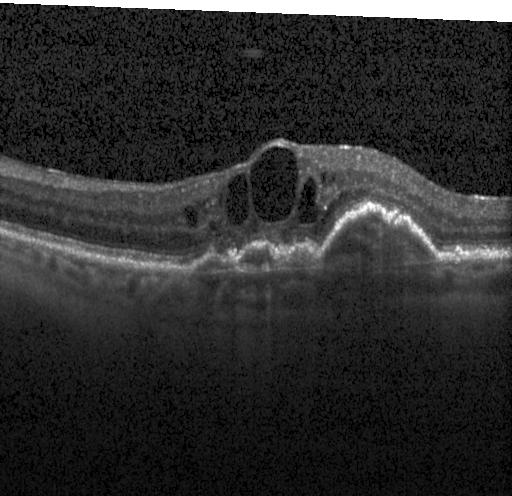 Heidelberg Spectralis; OCT B-scan; SD-OCT; macular scan.
Impression: choroidal neovascularization.